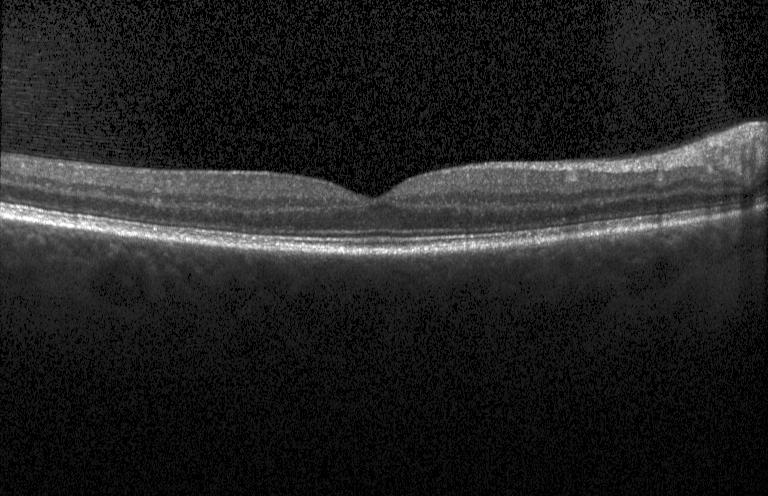
Retinal OCT B-scan · Heidelberg Spectralis OCT system · spectral-domain optical coherence tomography · fovea-centered. This B-scan demonstrates no evidence of choroidal neovascularization, diabetic macular edema, or drusen.